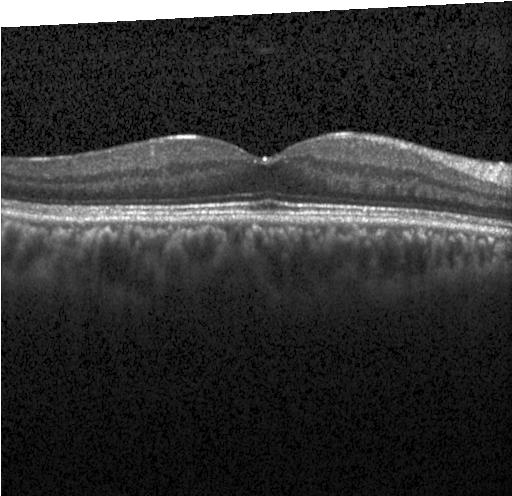

OCT B-scan.
This B-scan demonstrates no evidence of CNV, DME, or drusen.